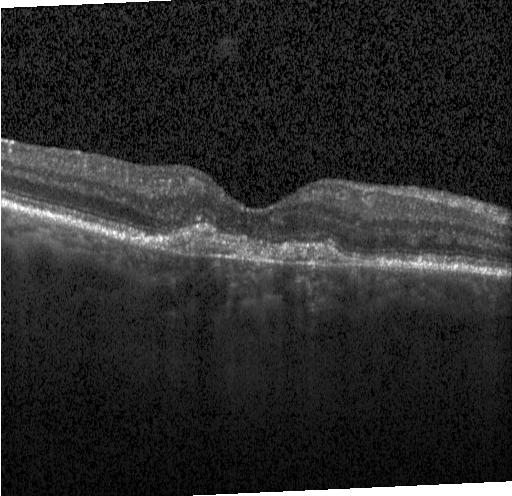 Optical coherence tomography B-scan, fovea-centered, SD-OCT.
Choroidal neovascularization.